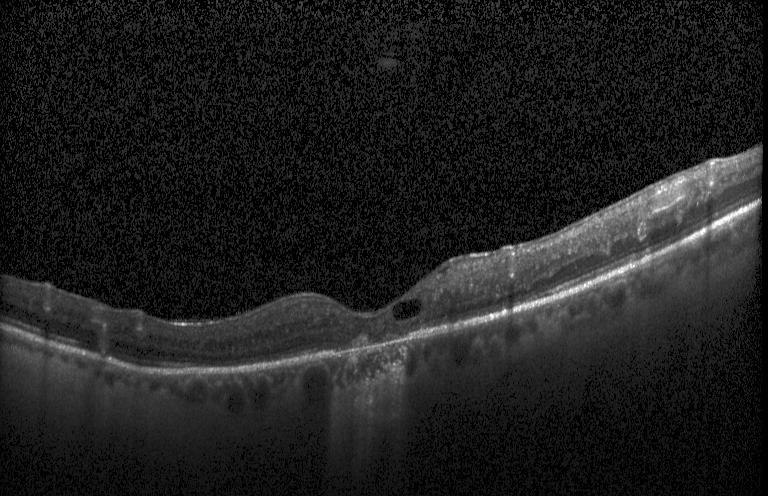

Finding: CNV.